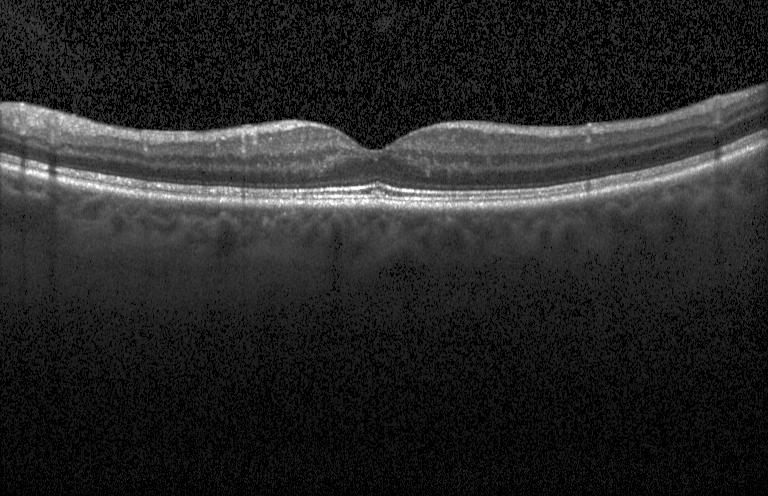
Retinal OCT cross-section · centered on the fovea.
Finding: no CNV, DME, or drusen.